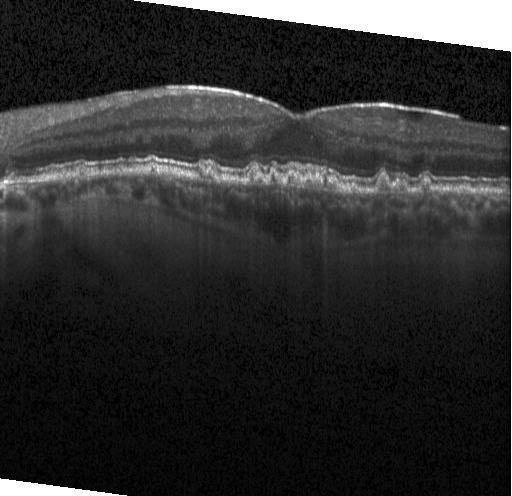
OCT line scan. Spectral-domain optical coherence tomography. Horizontal scan through the fovea. Heidelberg Spectralis OCT system. Macular OCT: drusen.